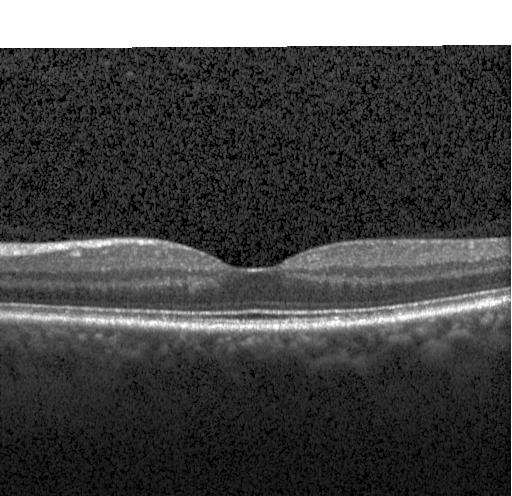
Retinal OCT B-scan
Assessment: no CNV, no DME, and no drusen.